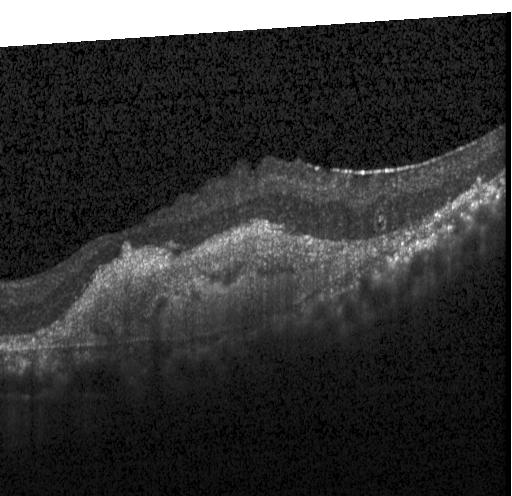
Spectral-domain optical coherence tomography, acquired on a Heidelberg Spectralis, horizontal scan through the fovea, OCT B-scan — This B-scan demonstrates a choroidal neovascular membrane.